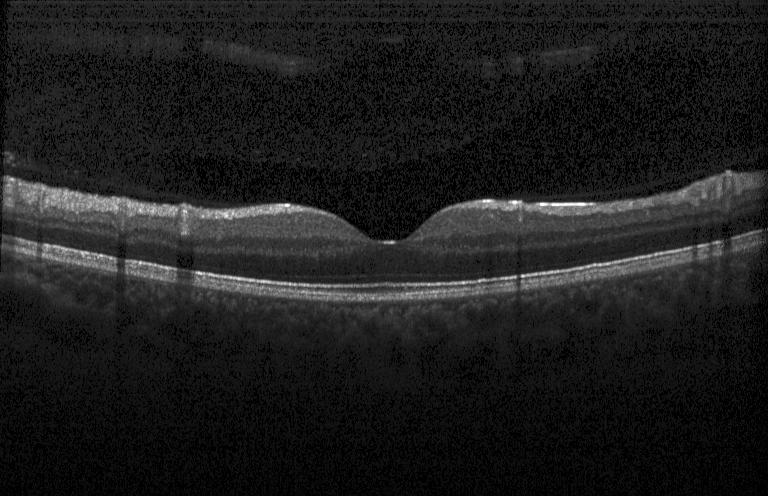 Dx: no evidence of CNV, DME, or drusen.